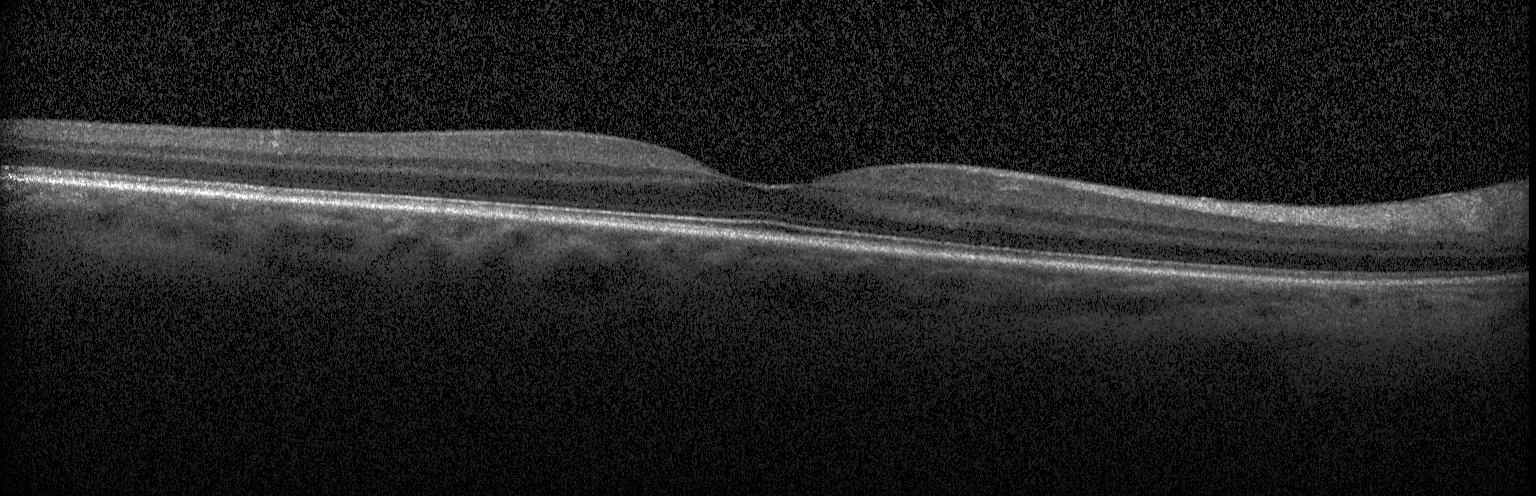
Centered on the fovea. Optical coherence tomography B-scan. SD-OCT.
This B-scan demonstrates no evidence of choroidal neovascularization, diabetic macular edema, or drusen.